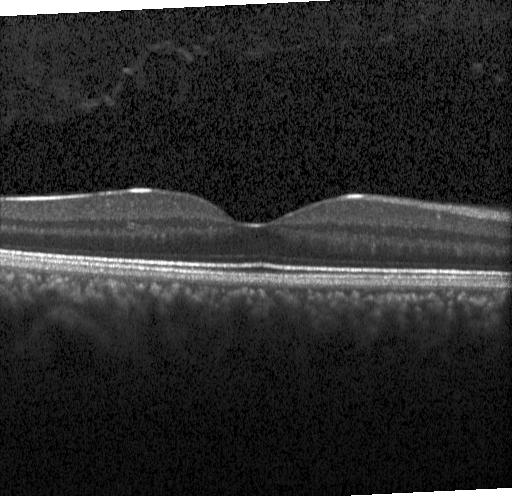 OCT B-scan.
Finding: no choroidal neovascularization, no diabetic macular edema, and no drusen.